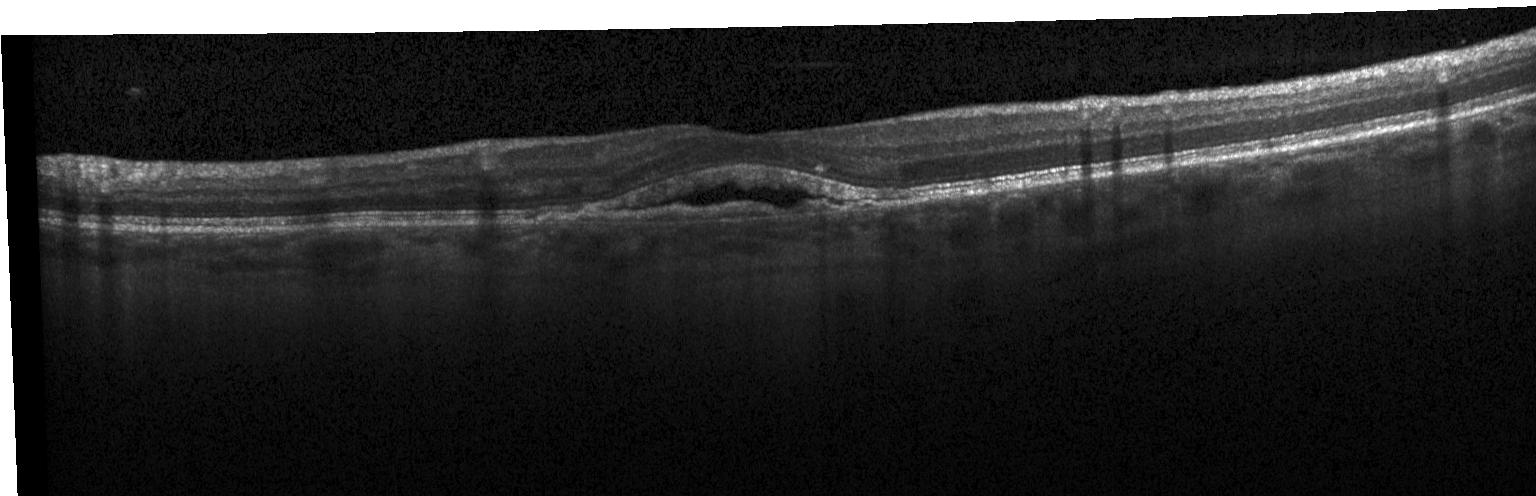

Heidelberg Spectralis OCT system · optical coherence tomography B-scan · macular scan
Finding: choroidal neovascularization.